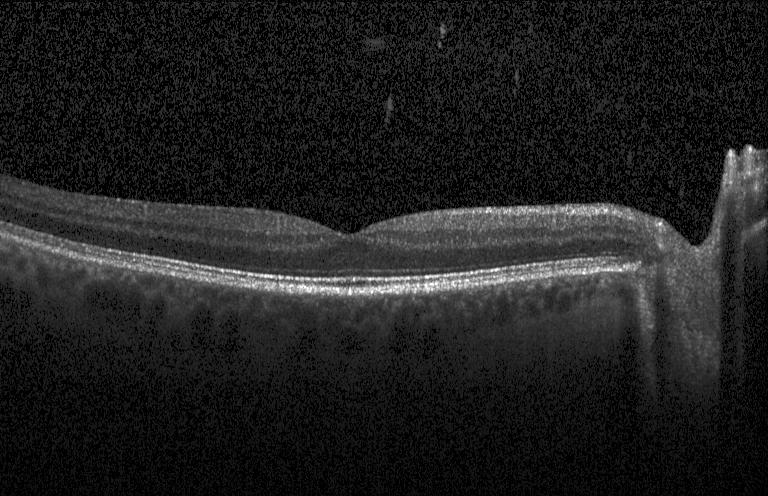
OCT line scan
Assessment: neither choroidal neovascularization, diabetic macular edema, nor drusen.